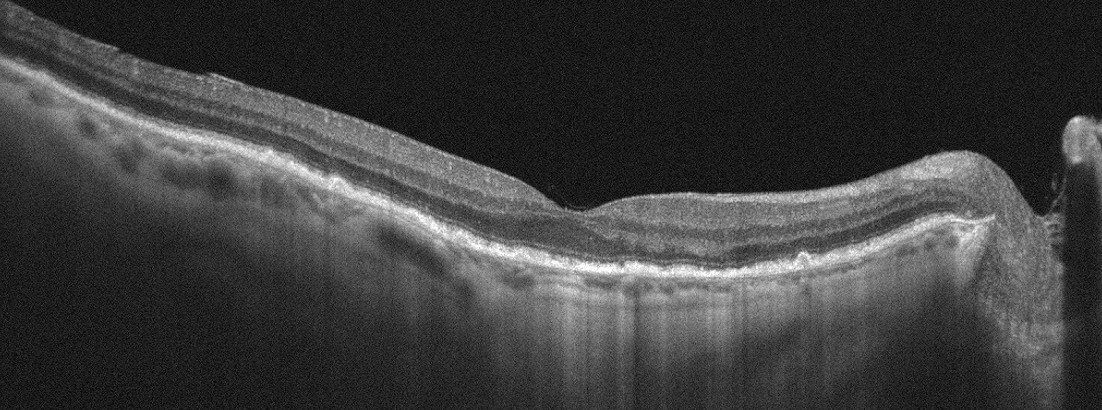
Optical coherence tomography B-scan — The scan shows age-related macular degeneration.